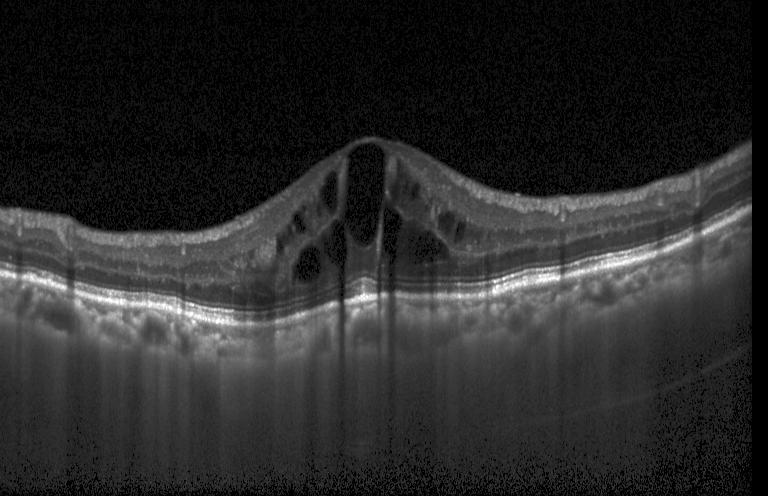

Spectral-domain OCT B-scan: diabetic macular edema.